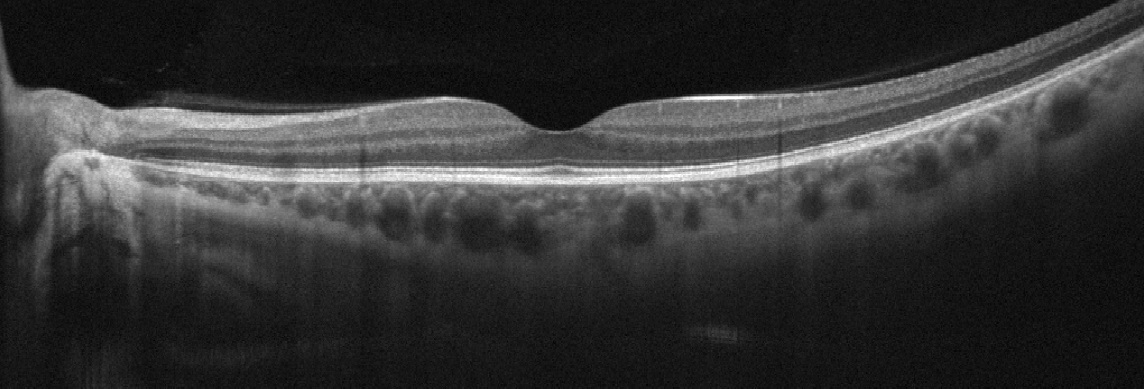
The scan shows no AMD, DME, ERM, RAO, RVO, or VID.